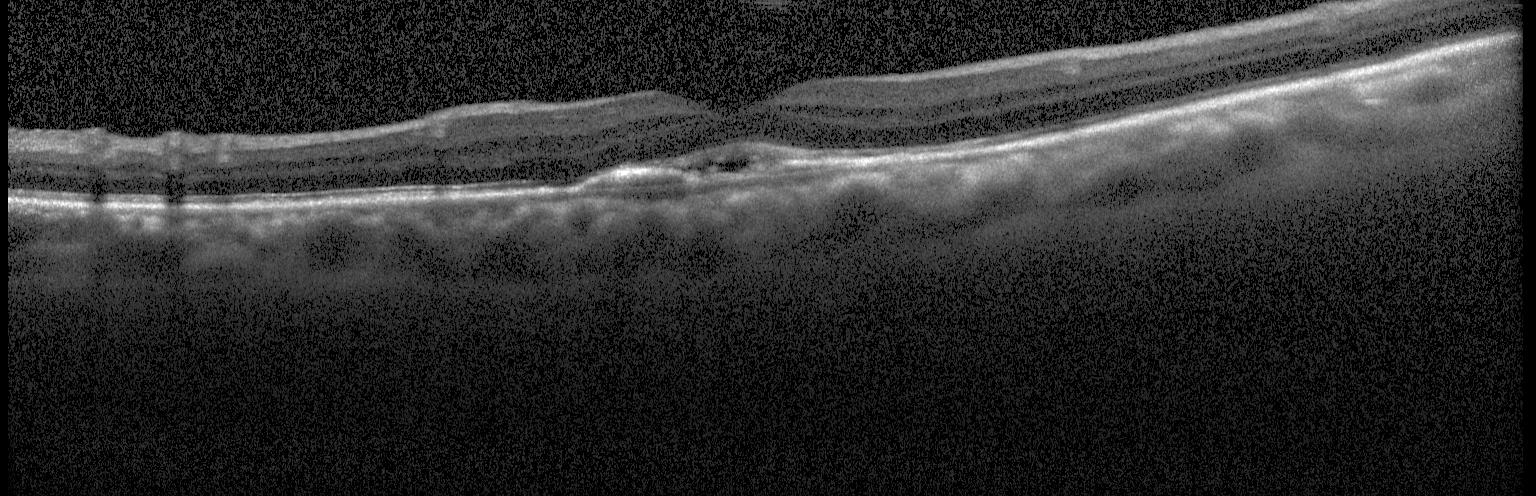 OCT scan showing a choroidal neovascular membrane.